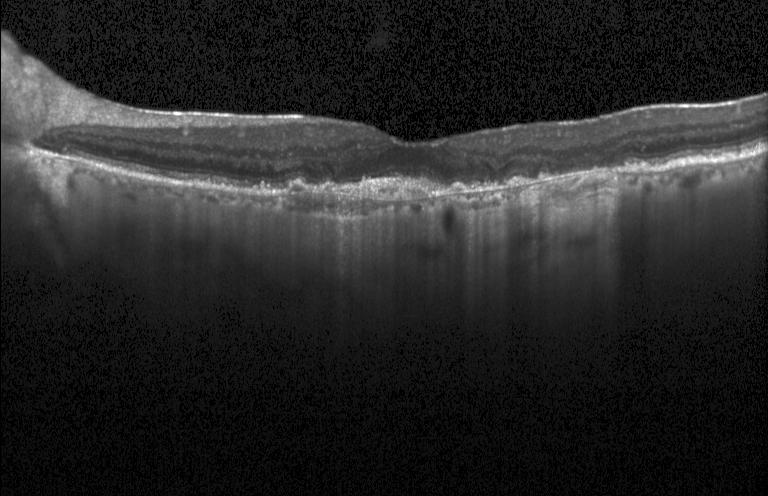 Macular OCT demonstrating choroidal neovascularization.